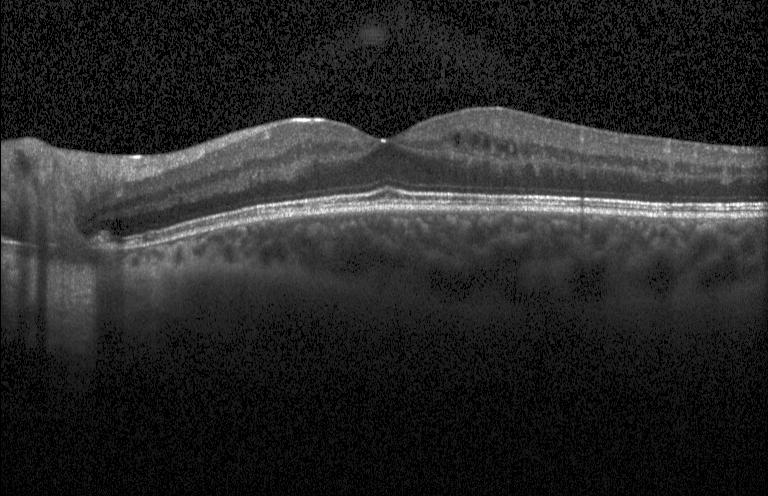
This B-scan demonstrates diabetic macular edema (DME).